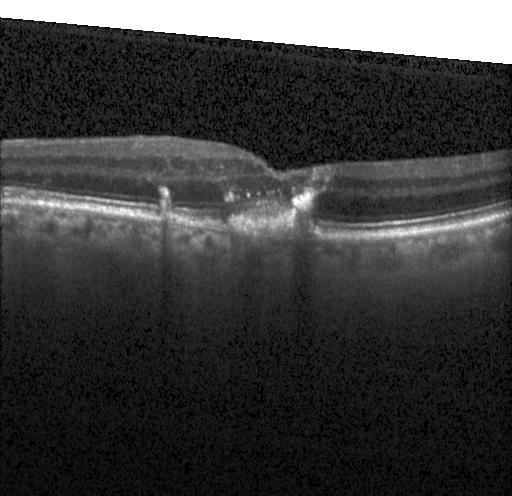

Spectral-domain OCT · Heidelberg Spectralis OCT system · OCT line scan · centered on the fovea
Macular OCT: choroidal neovascularization.